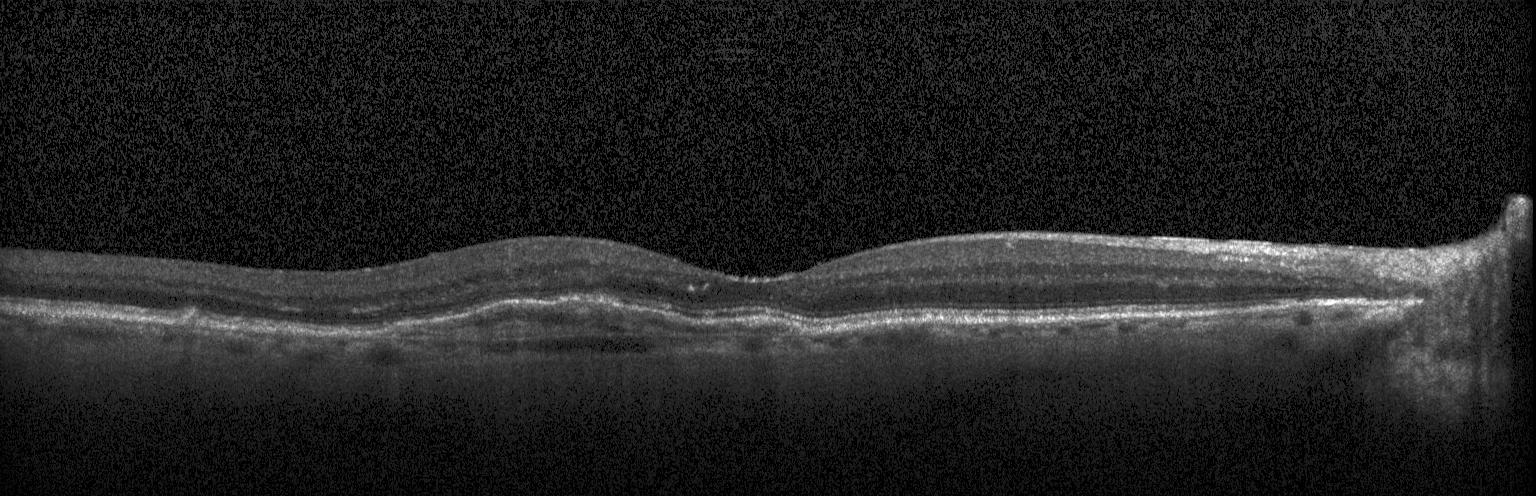 Optical coherence tomography scan, horizontal scan through the fovea, Heidelberg Spectralis, spectral-domain OCT. A choroidal neovascular membrane.